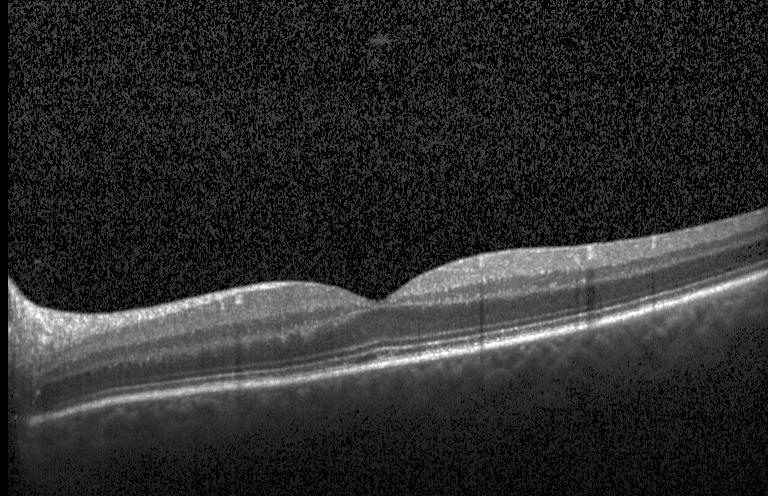

Optical coherence tomography B-scan · macular scan · Heidelberg Spectralis OCT system. Macular OCT: no choroidal neovascularization, no diabetic macular edema, and no drusen.